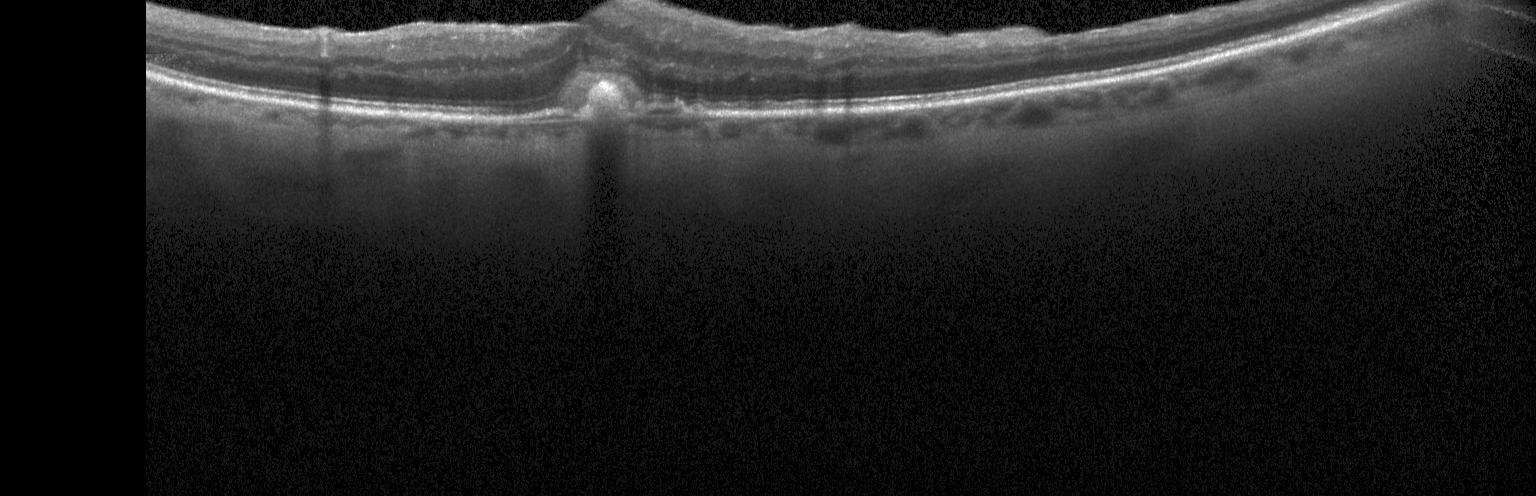

Spectral-domain optical coherence tomography. Retinal OCT cross-section. Impression: choroidal neovascularization (CNV).